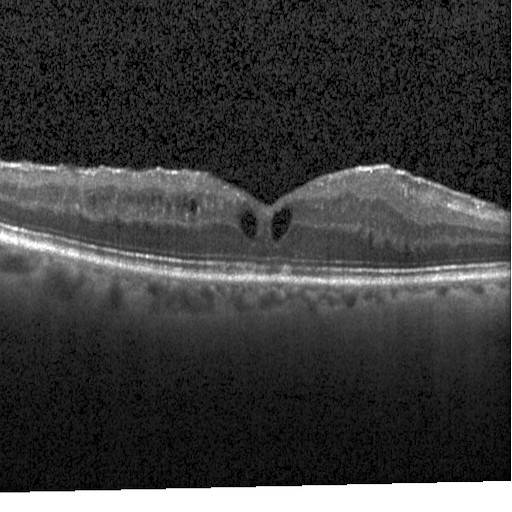 Optical coherence tomography scan, horizontal scan through the fovea
The scan shows DME.